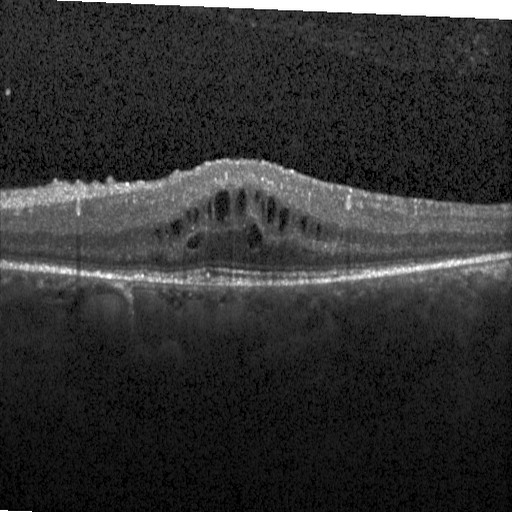

Fovea-centered; spectral-domain OCT; retinal OCT B-scan; instrument: Heidelberg Spectralis.
Diagnosis: diabetic macular edema (DME).